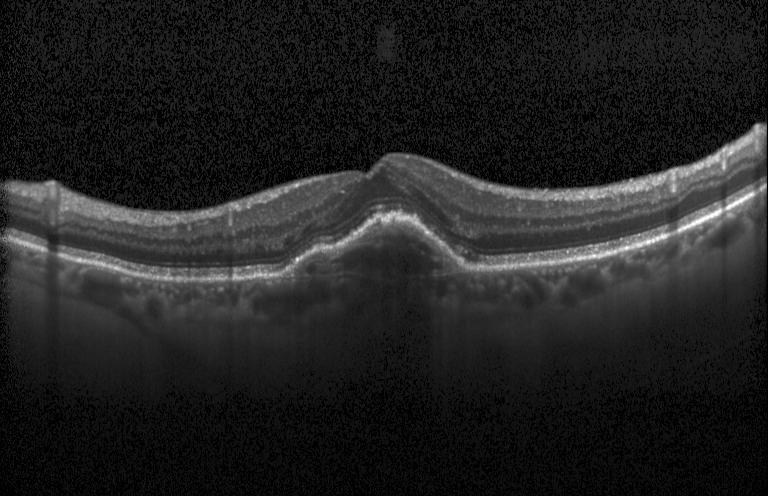 Spectral-domain OCT. Centered on the fovea. Optical coherence tomography B-scan.
Finding: a choroidal neovascular membrane.